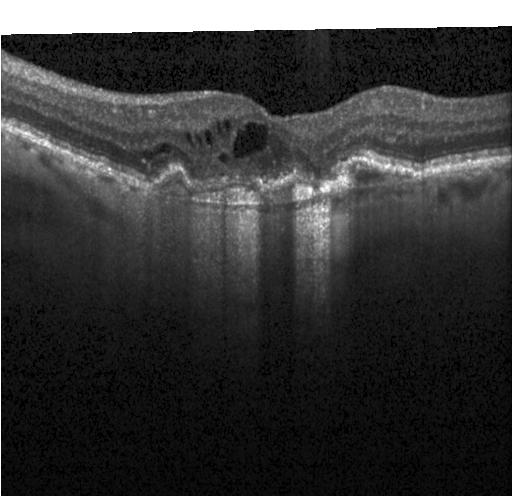

Retinal OCT cross-section, SD-OCT
The scan shows CNV.